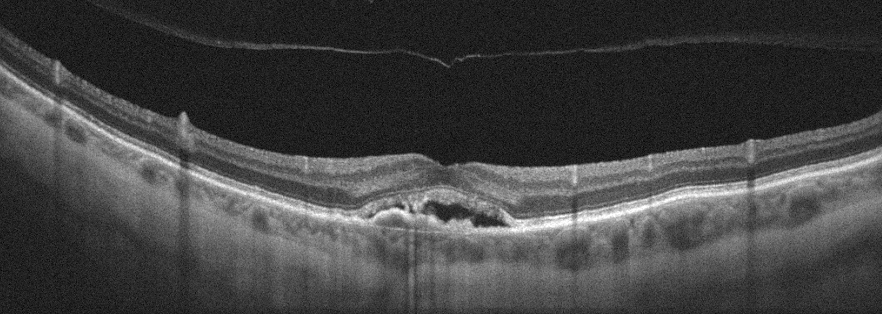 Acquired on an Optovue Avanti RTVue XR. Retinal OCT cross-section. Left eye. Fovea-centered
Finding: age-related macular degeneration (AMD).